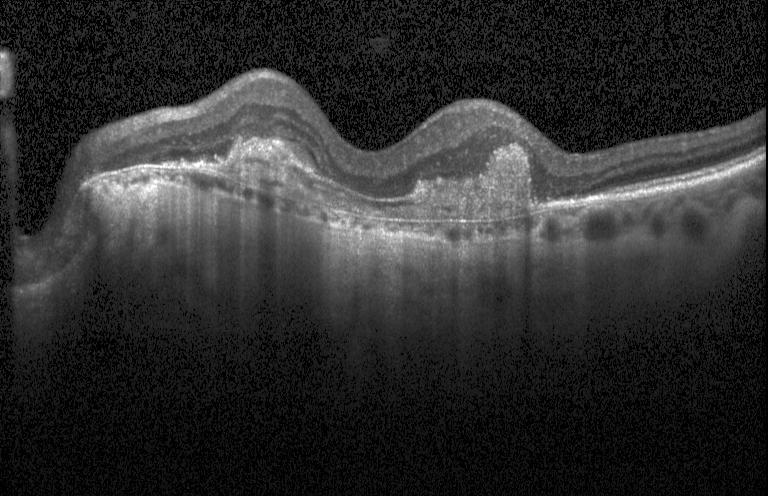 Optical coherence tomography B-scan. Fovea-centered
Assessment: a choroidal neovascular membrane.